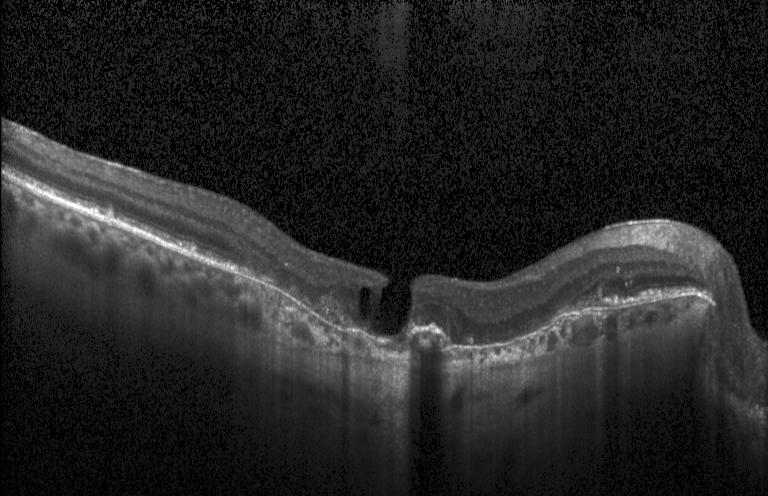
OCT B-scan showing choroidal neovascularization.